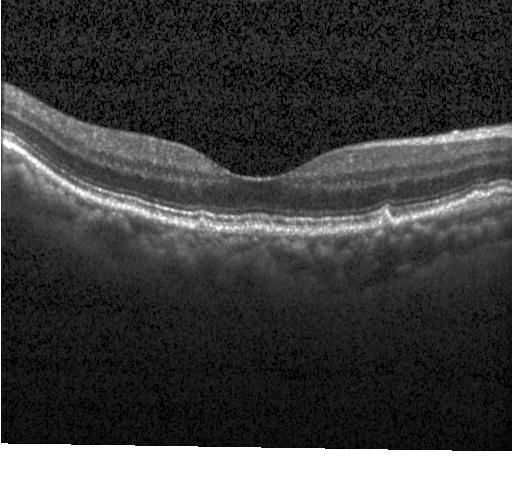 SD-OCT, optical coherence tomography B-scan, macular scan
Impression: multiple drusen.